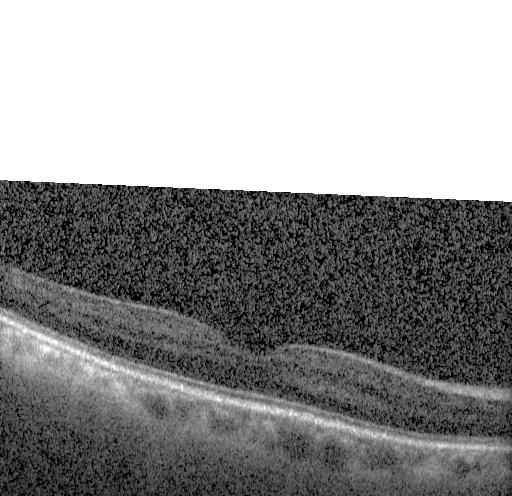 Retinal OCT cross-section; acquired on a Heidelberg Spectralis; spectral-domain OCT
Finding: no choroidal neovascularization, no diabetic macular edema, and no drusen.